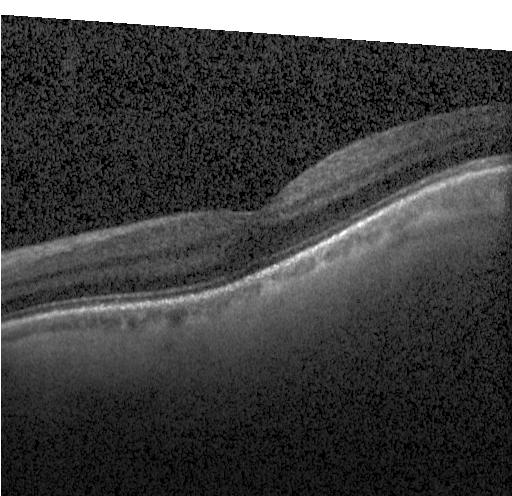
Instrument: Heidelberg Spectralis, SD-OCT, retinal OCT cross-section
This B-scan demonstrates no choroidal neovascularization, no diabetic macular edema, and no drusen.